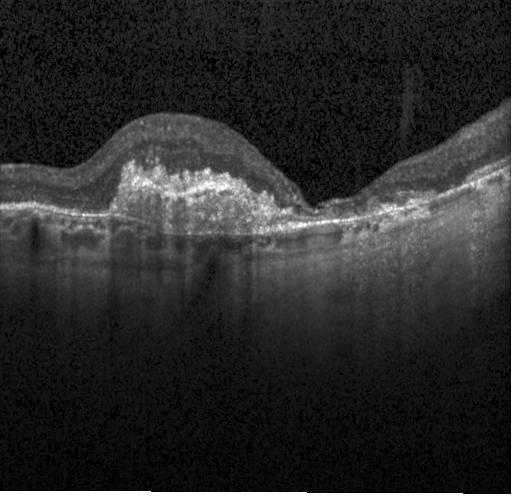
Fovea-centered; SD-OCT; optical coherence tomography scan; acquired on a Heidelberg Spectralis
Diagnosis: a choroidal neovascular membrane.